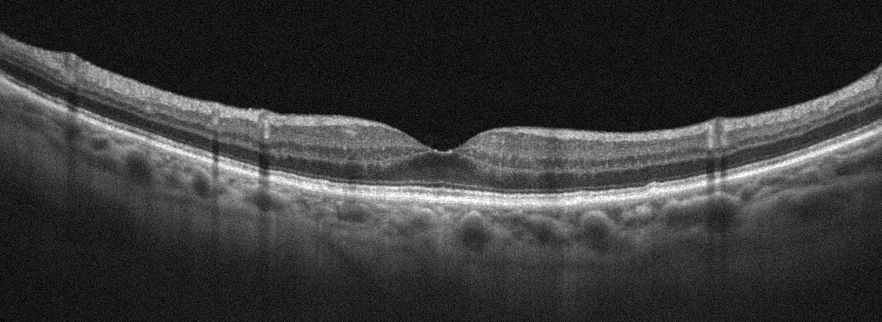

Oculus sinister. Optical coherence tomography scan.
Dx: age-related macular degeneration.